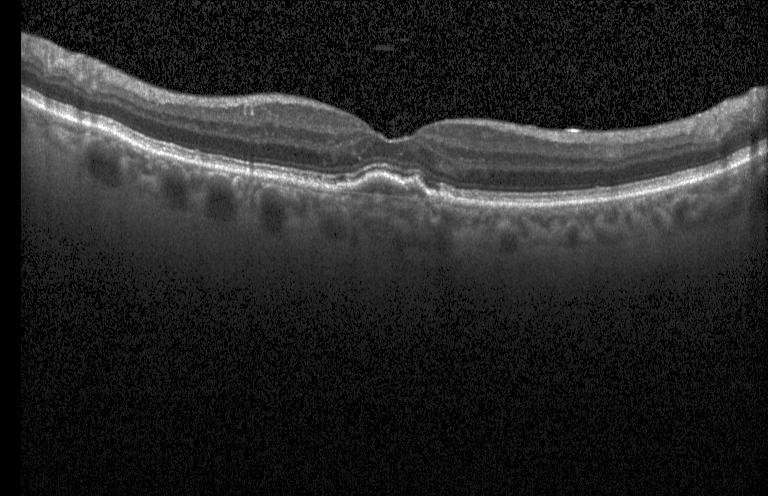 Centered on the fovea, OCT B-scan.
This B-scan demonstrates a choroidal neovascular membrane.